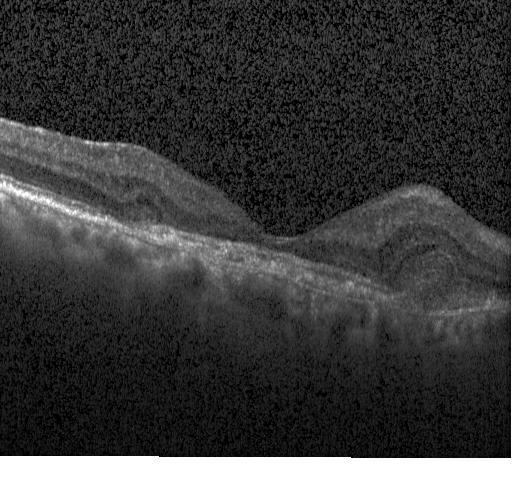

Retinal OCT B-scan
Impression: a choroidal neovascular membrane.